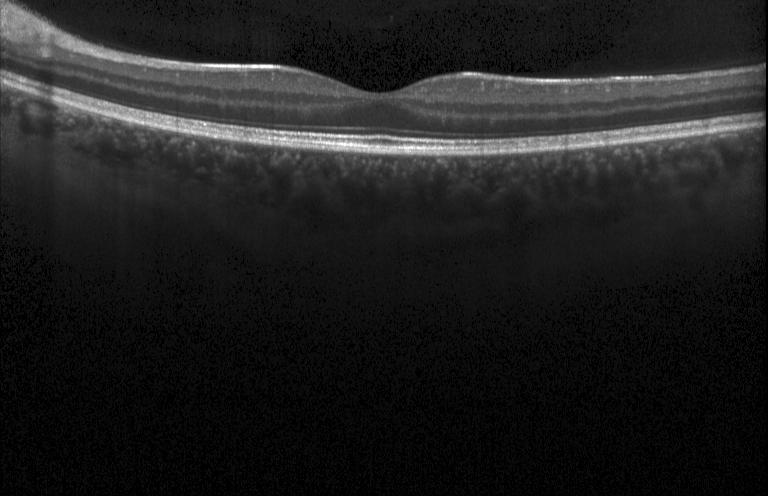

Spectral-domain OCT. Instrument: Heidelberg Spectralis. Retinal OCT cross-section. Centered on the fovea — Impression: no choroidal neovascularization, no diabetic macular edema, and no drusen.